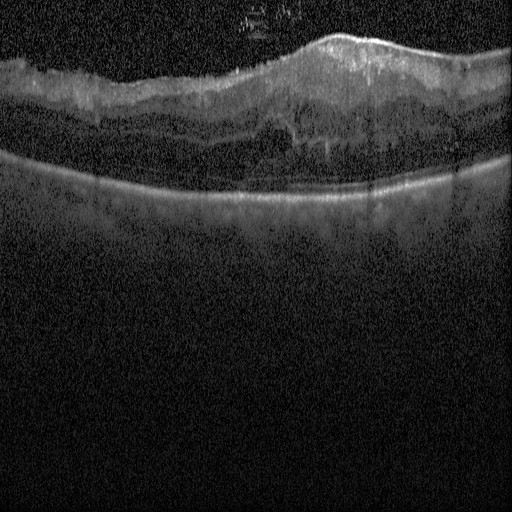 Through the macula. Instrument: Heidelberg Spectralis. OCT B-scan. SD-OCT
Diagnosis: diabetic macular edema.